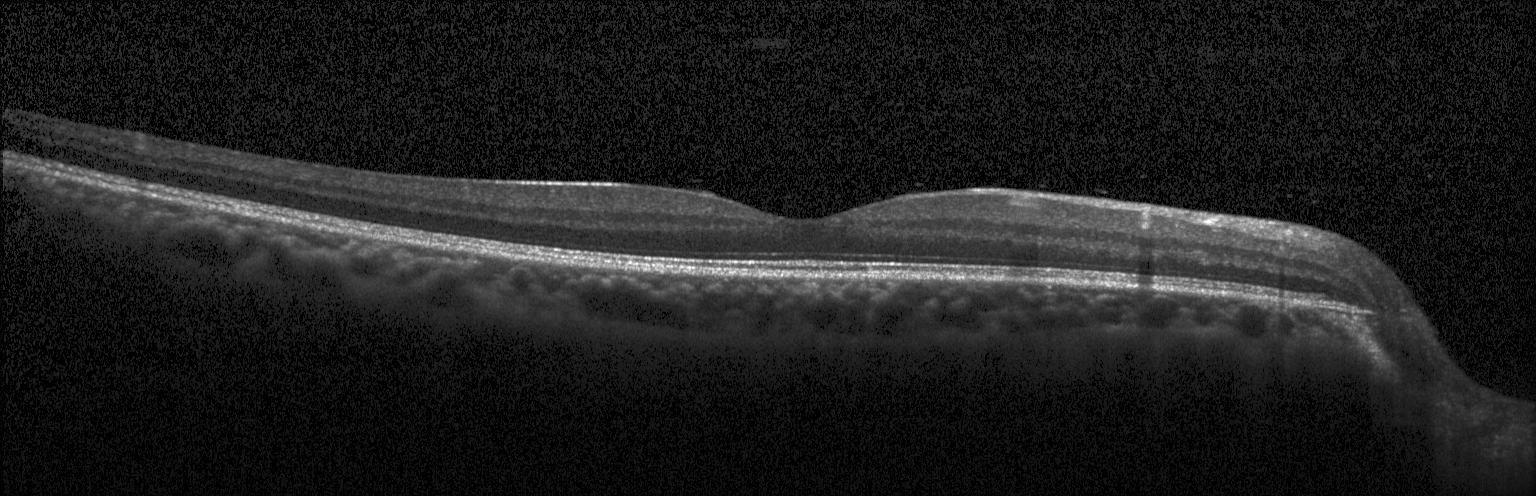
OCT B-scan showing no evidence of choroidal neovascularization, diabetic macular edema, or drusen.